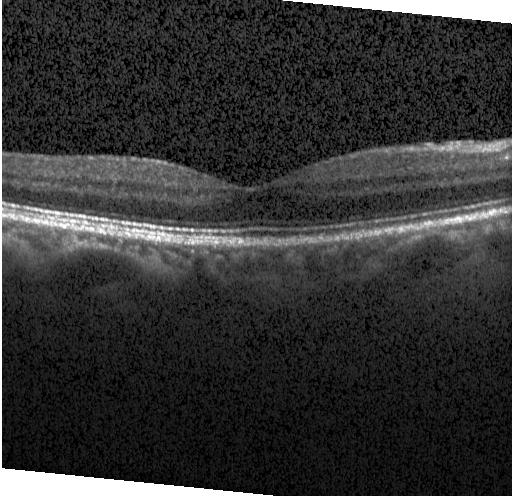 Optical coherence tomography B-scan, fovea-centered, SD-OCT, instrument: Heidelberg Spectralis — Impression: no choroidal neovascularization, diabetic macular edema, or drusen.